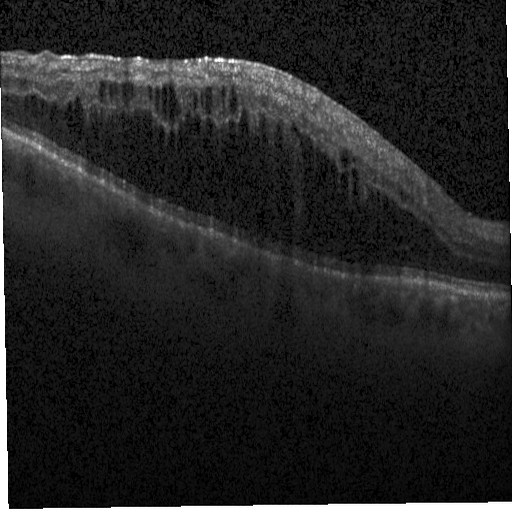
Finding: diabetic macular edema.